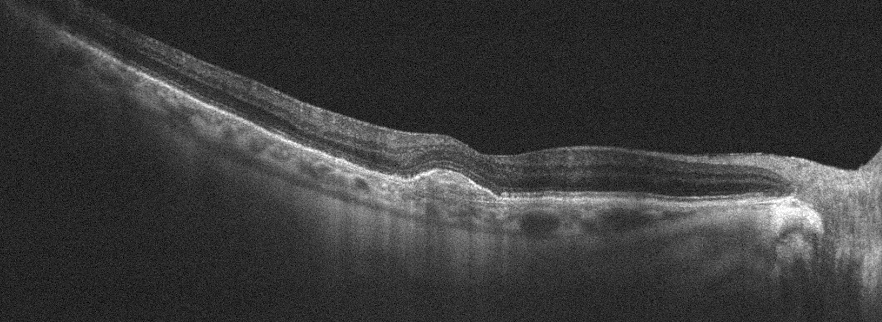 Dx: age-related macular degeneration (AMD).